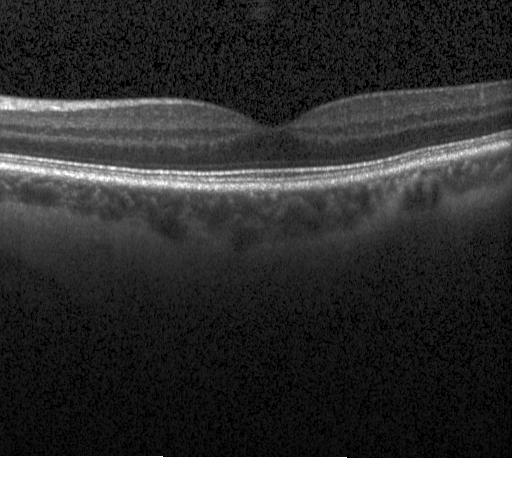

Dx: no evidence of CNV, DME, or drusen.